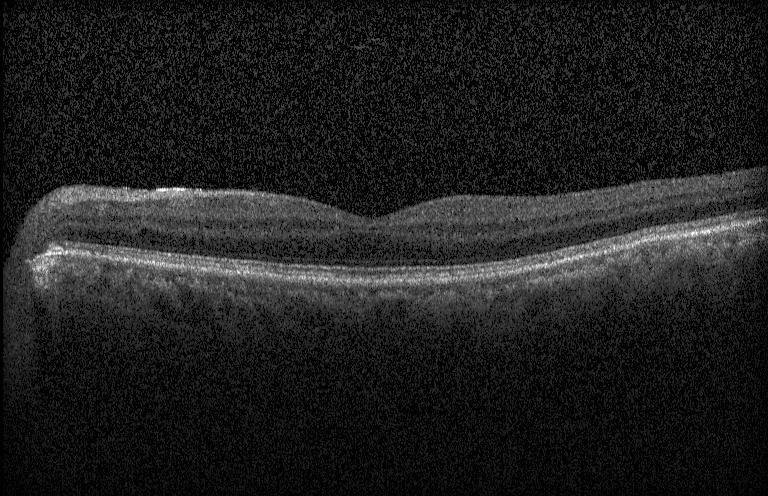
Heidelberg Spectralis OCT system; through the macula; spectral-domain optical coherence tomography; retinal OCT cross-section — Dx: no evidence of choroidal neovascularization, diabetic macular edema, or drusen.